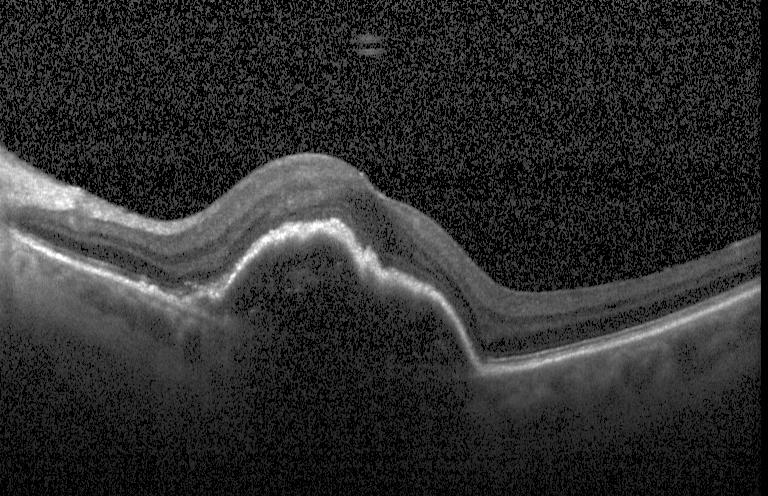
Assessment: CNV.